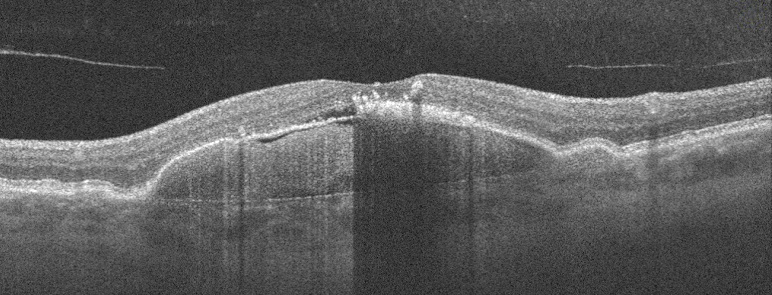 Instrument: Optovue Avanti RTVue XR; retinal OCT cross-section.
Finding: age-related macular degeneration (AMD).